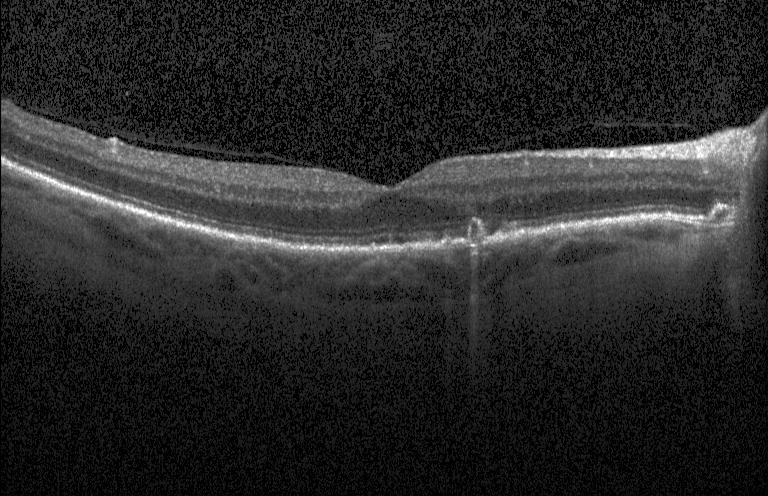

OCT B-scan.
The scan shows drusen.